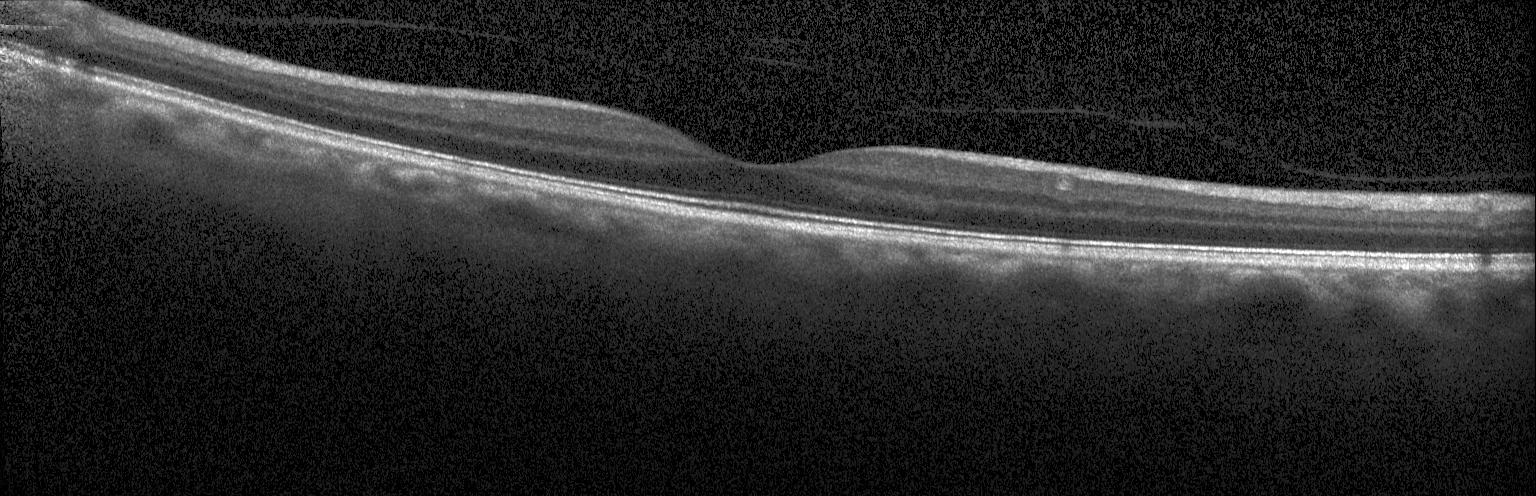 Optical coherence tomography scan; Heidelberg Spectralis; through the macula; SD-OCT — Diagnosis: no CNV, no DME, and no drusen.